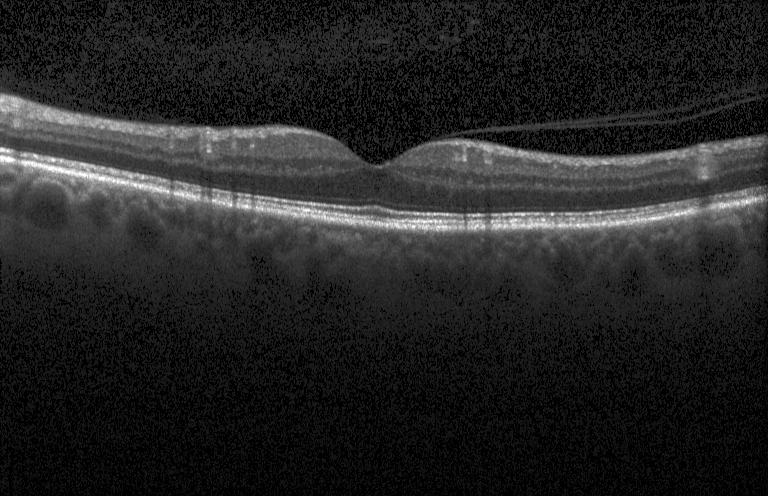

Finding: no choroidal neovascularization, diabetic macular edema, or drusen.